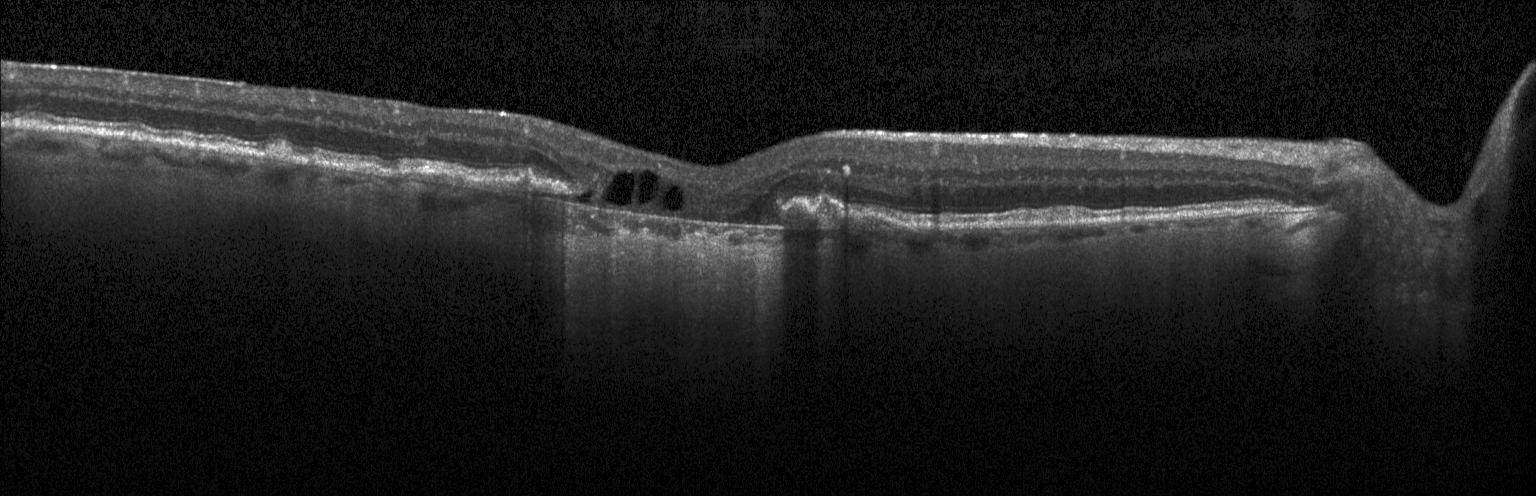

Impression: choroidal neovascularization (CNV).